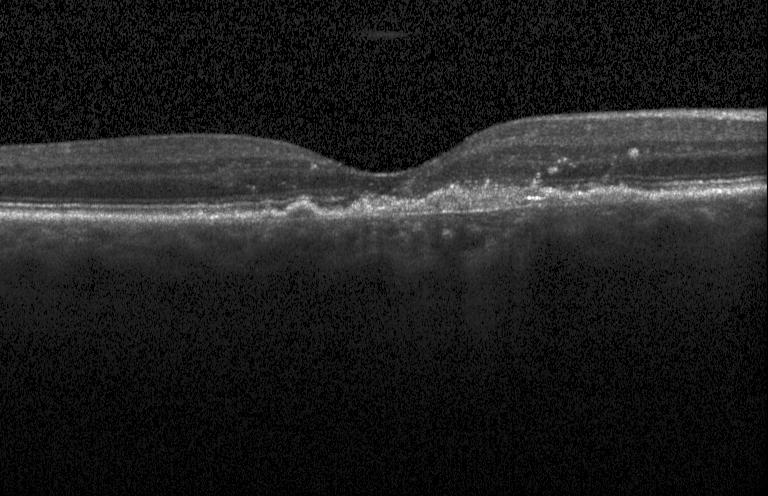
Heidelberg Spectralis OCT system · optical coherence tomography scan
Impression: choroidal neovascularization.